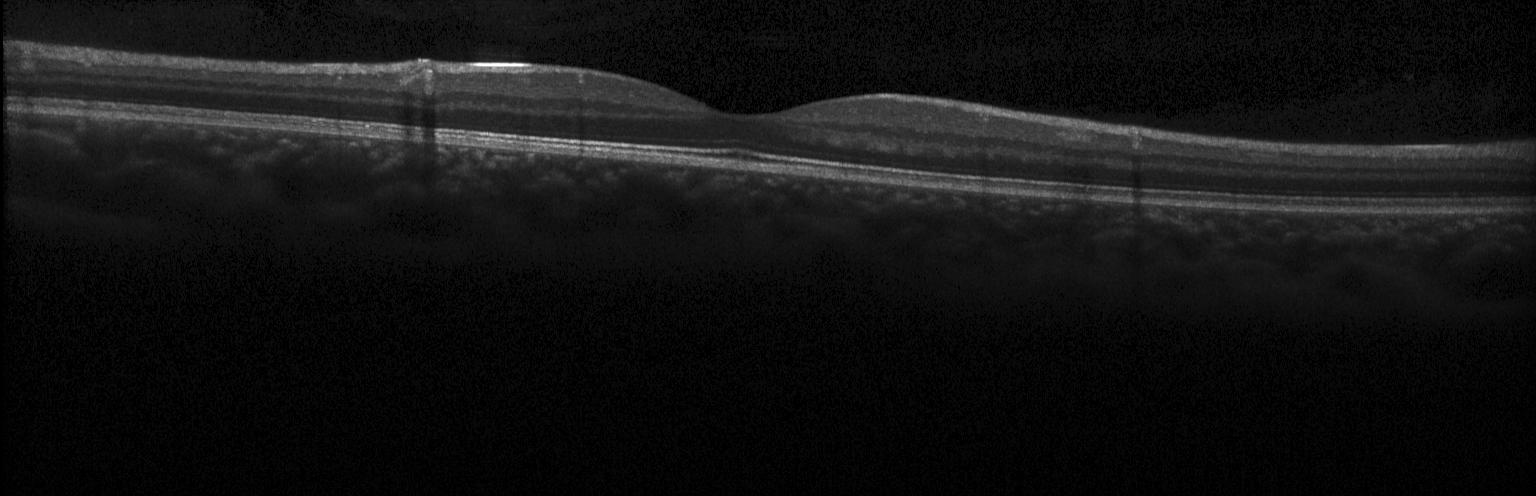

Finding: no CNV, no DME, and no drusen.